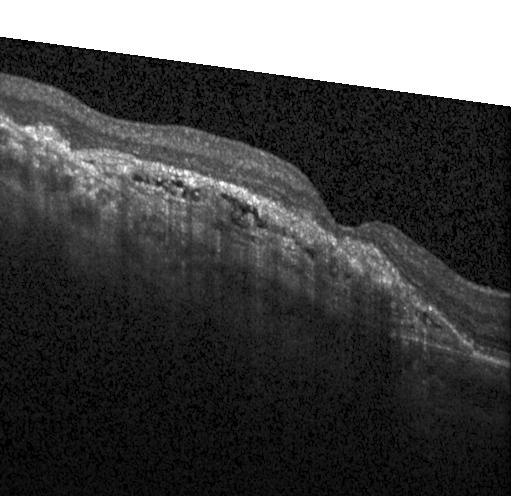 Optical coherence tomography scan · spectral-domain OCT · Heidelberg Spectralis · through the macula — Impression: a choroidal neovascular membrane.